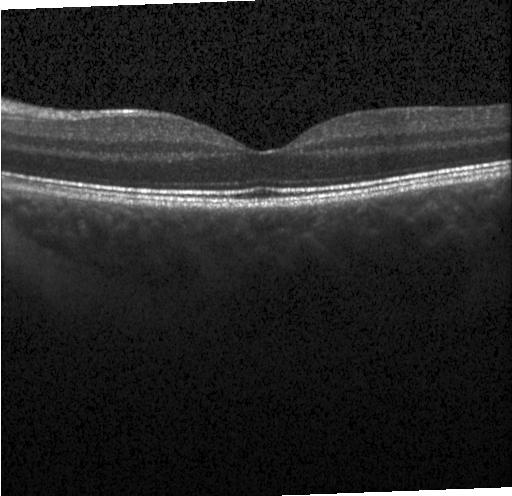
Retinal OCT cross-section — Finding: no choroidal neovascularization, no diabetic macular edema, and no drusen.